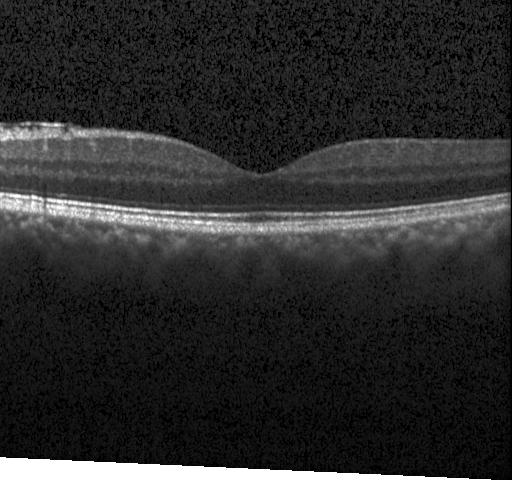 Macular OCT: no choroidal neovascularization, no diabetic macular edema, and no drusen.